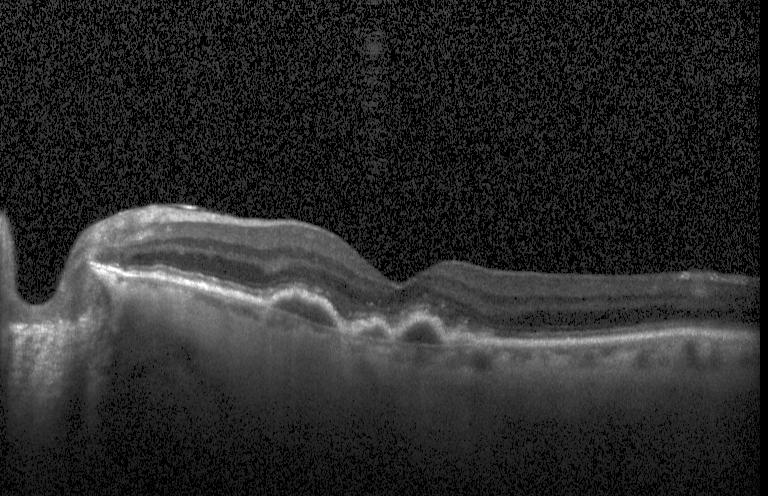 Spectral-domain OCT · horizontal scan through the fovea · retinal OCT B-scan. Finding: a choroidal neovascular membrane.